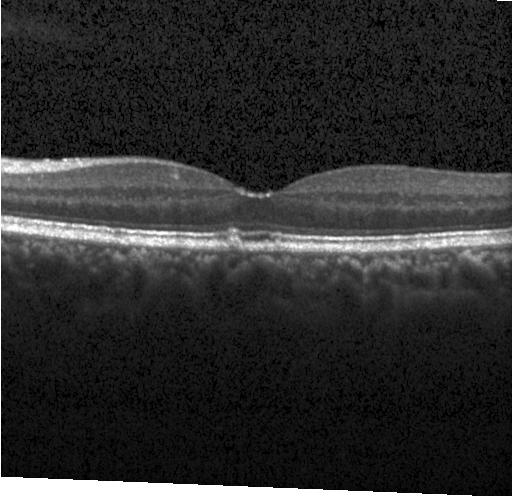

SD-OCT · Heidelberg Spectralis OCT system · macular scan · optical coherence tomography B-scan. Finding: drusen.